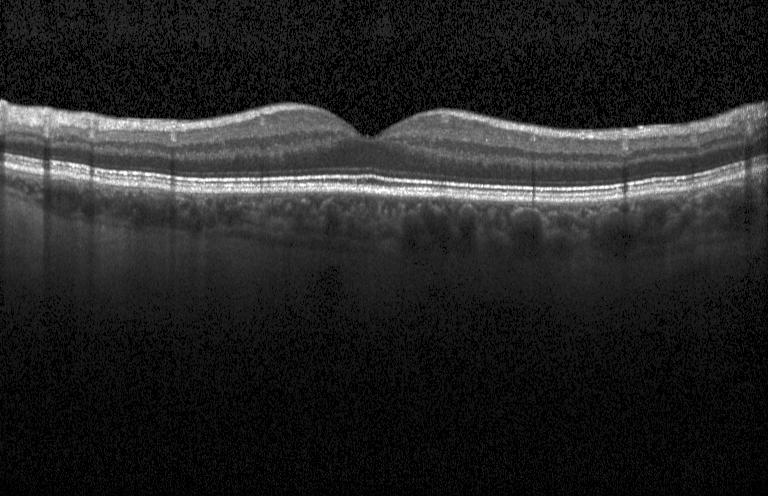 Spectral-domain OCT B-scan: no choroidal neovascularization, diabetic macular edema, or drusen.